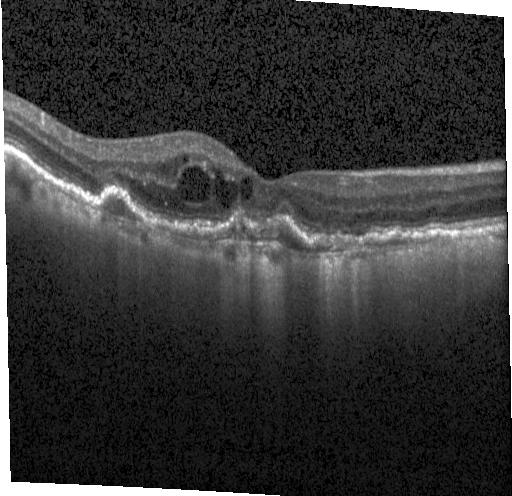
Spectral-domain optical coherence tomography, OCT line scan, Heidelberg Spectralis OCT system.
Finding: choroidal neovascularization (CNV).